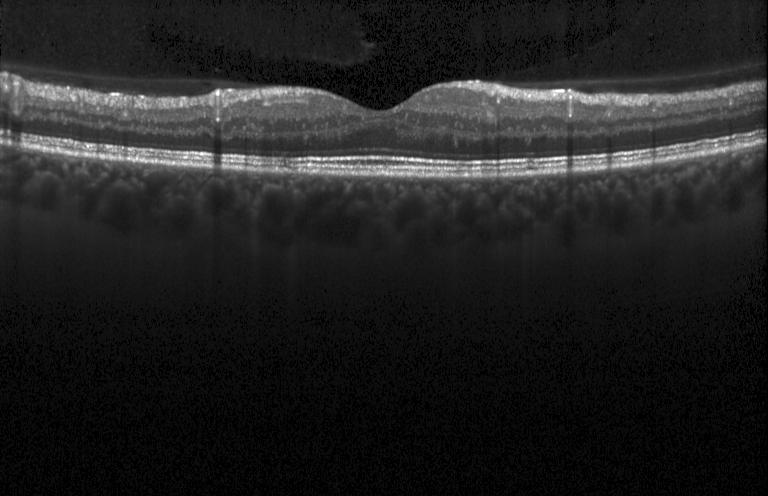

Instrument: Heidelberg Spectralis, OCT B-scan
This B-scan demonstrates no CNV, DME, or drusen.